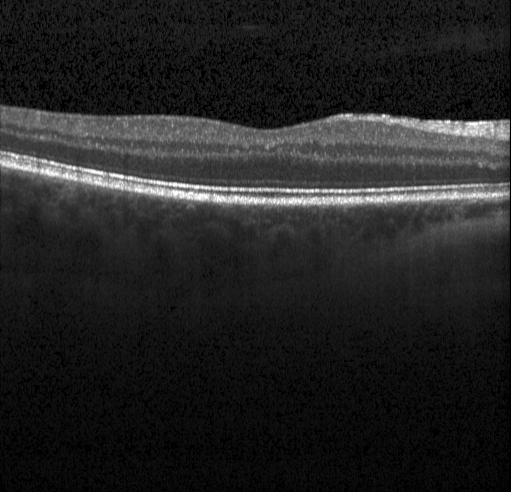
Diagnosis: neither choroidal neovascularization, diabetic macular edema, nor drusen.